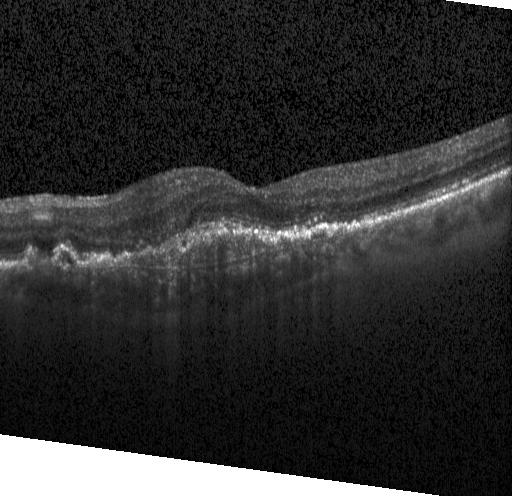
OCT line scan.
Diagnosis: choroidal neovascularization.